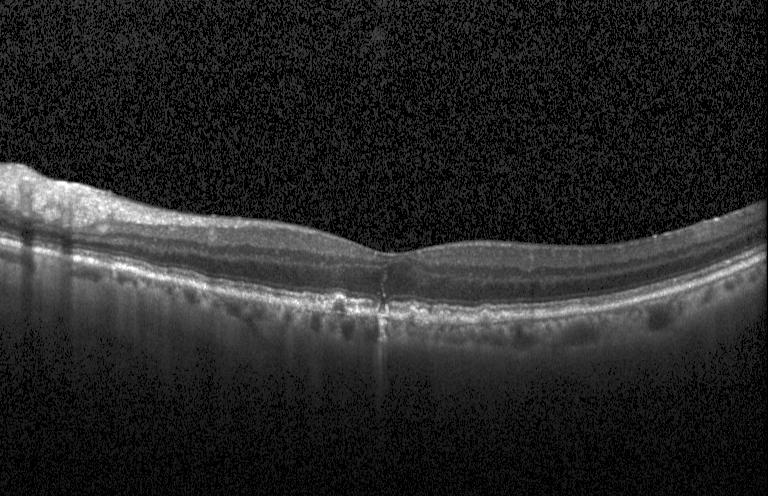

Retinal OCT cross-section showing multiple drusen.